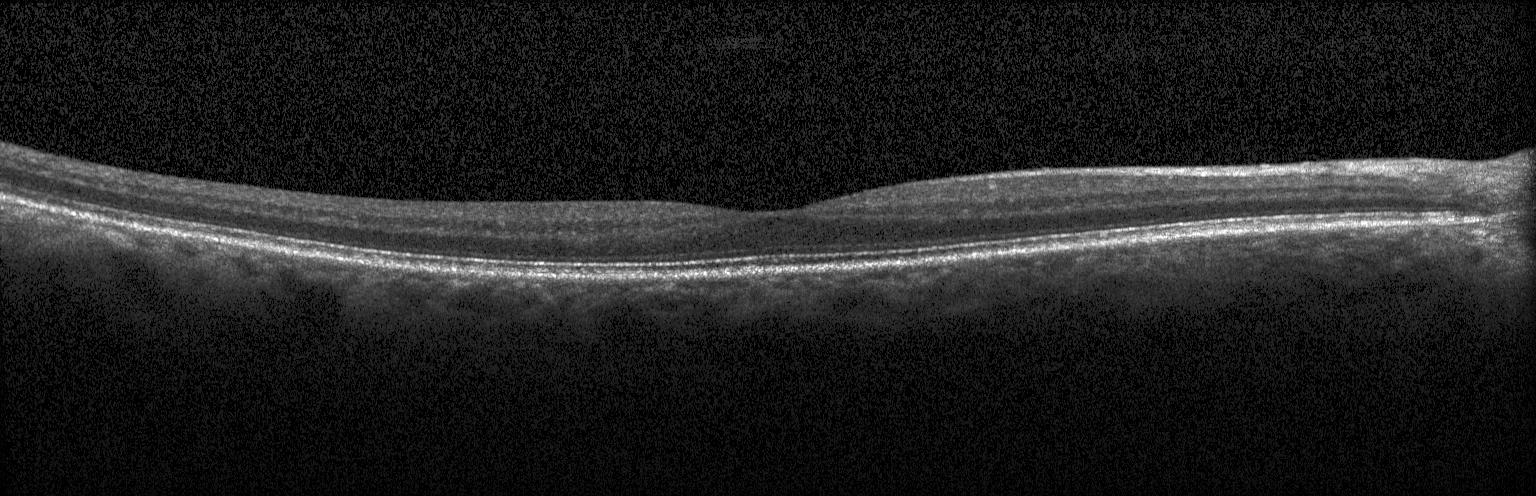

Retinal OCT cross-section. Through the macula. SD-OCT. Assessment: no CNV, DME, or drusen.